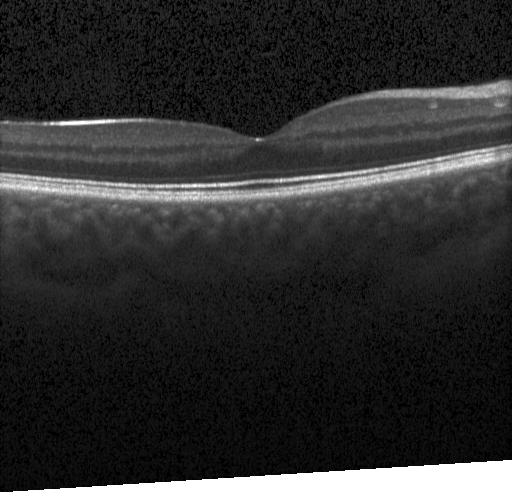 Spectral-domain OCT B-scan: no CNV, DME, or drusen.